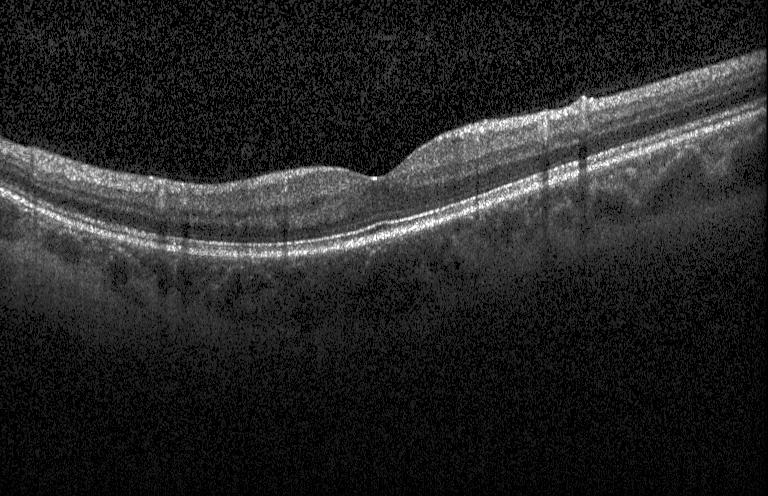 The scan shows no CNV, DME, or drusen.